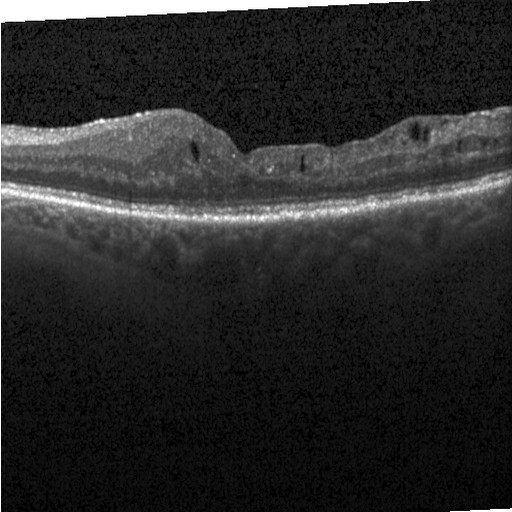
Dx: diabetic macular edema (DME).